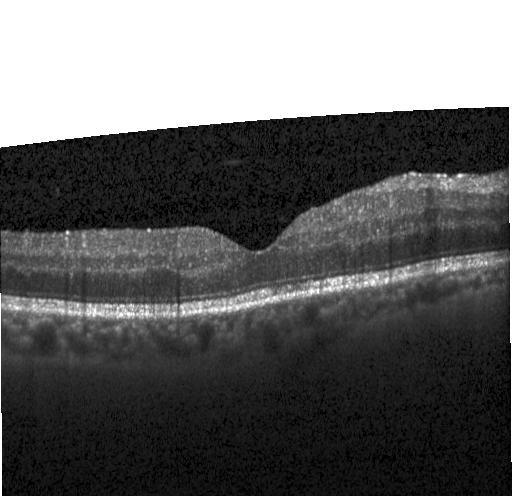 OCT finding: no choroidal neovascularization, diabetic macular edema, or drusen.